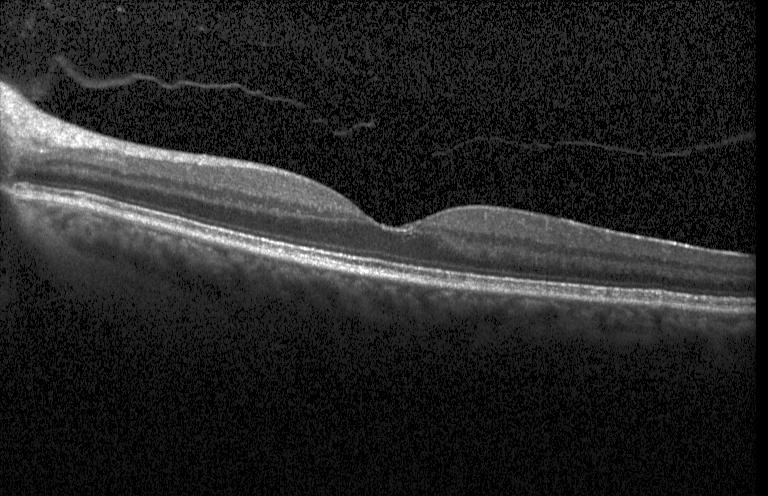
Horizontal scan through the fovea. Heidelberg Spectralis. OCT B-scan. SD-OCT.
OCT finding: no CNV, DME, or drusen.